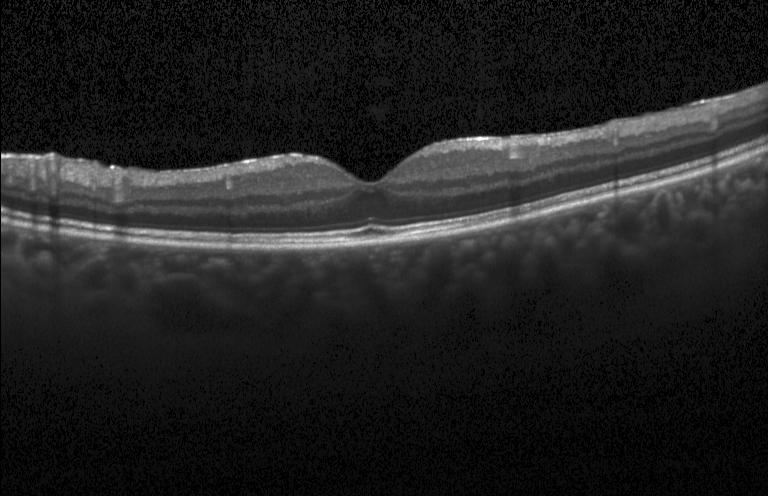
No choroidal neovascularization, diabetic macular edema, or drusen.